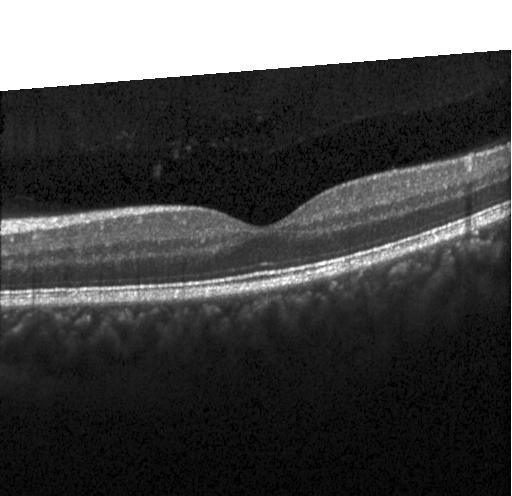

Diagnosis: no evidence of choroidal neovascularization, diabetic macular edema, or drusen.